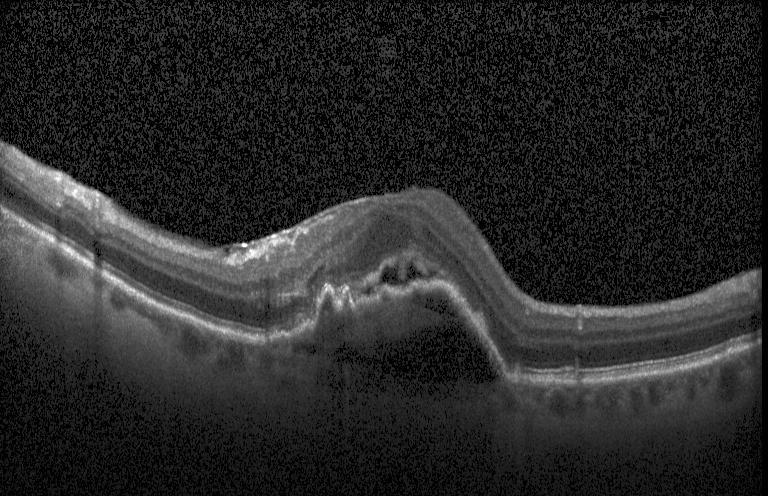
The scan shows choroidal neovascularization.